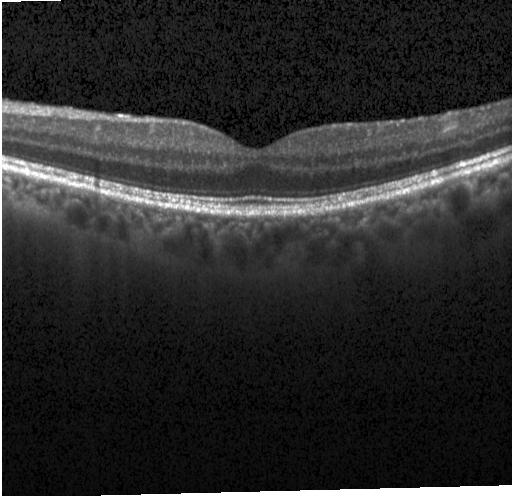

OCT line scan · spectral-domain OCT · through the macula — Macular OCT: neither CNV, DME, nor drusen.